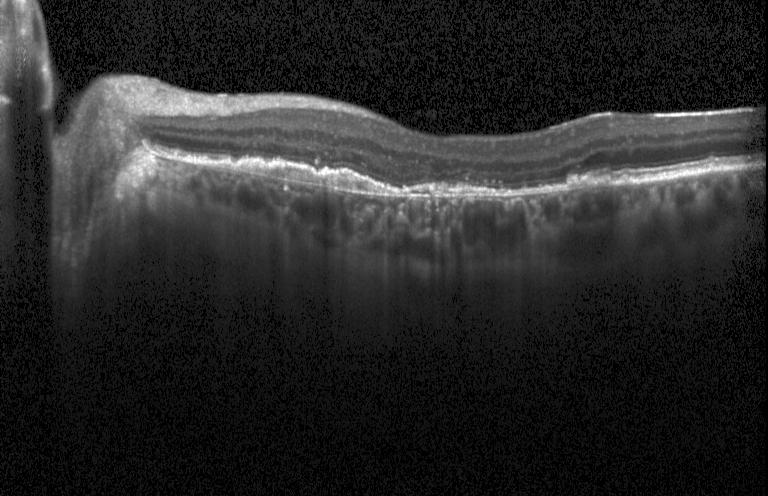
Spectral-domain OCT, OCT line scan — The scan shows CNV.